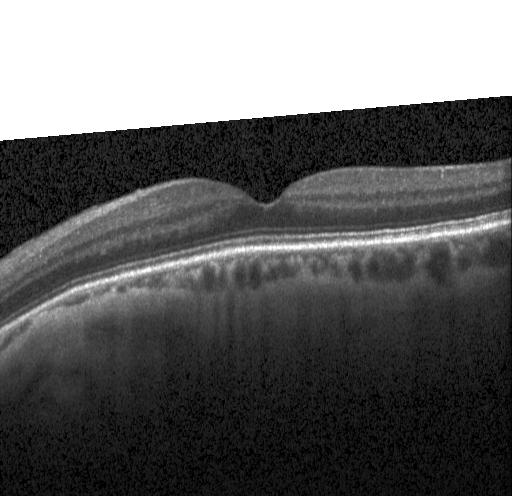 OCT finding: no choroidal neovascularization, no diabetic macular edema, and no drusen.